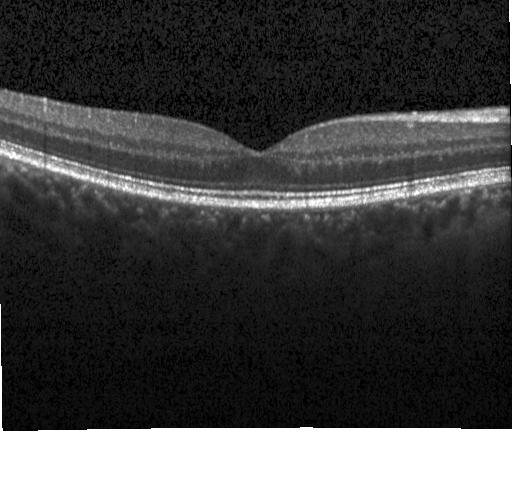 Spectral-domain optical coherence tomography; acquired on a Heidelberg Spectralis; retinal OCT cross-section — No evidence of choroidal neovascularization, diabetic macular edema, or drusen.